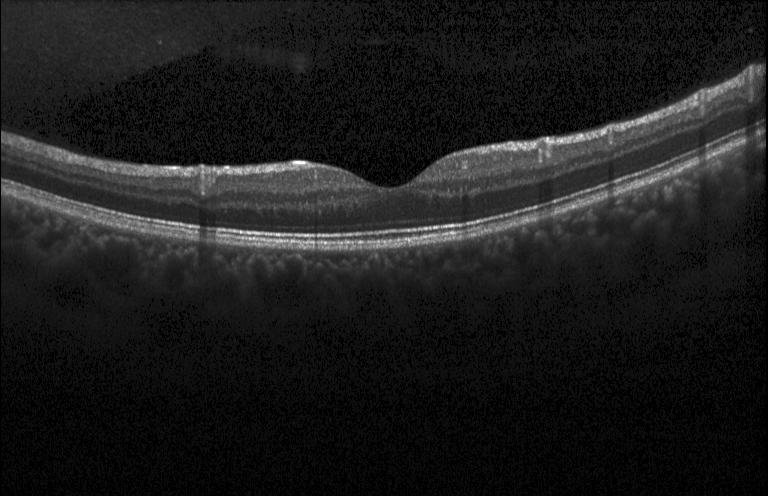 Impression: no CNV, no DME, and no drusen.